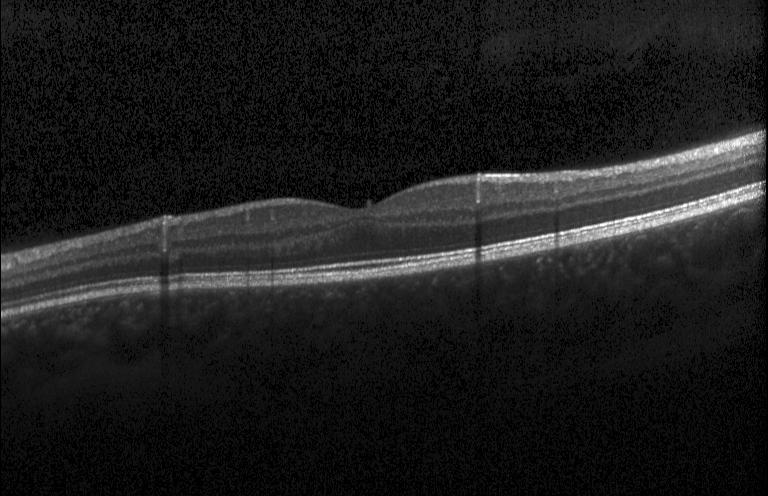
OCT scan showing no CNV, DME, or drusen.